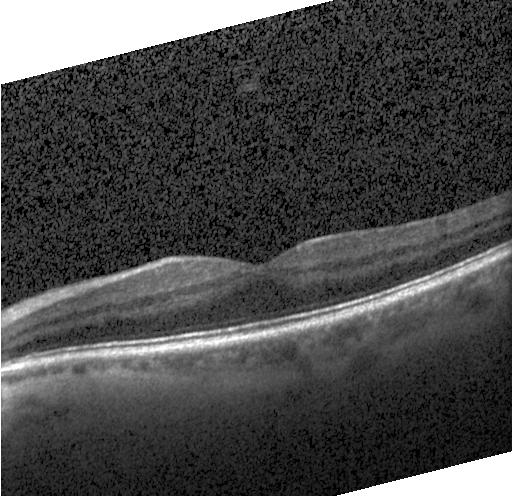
Retinal OCT B-scan. No CNV, DME, or drusen.